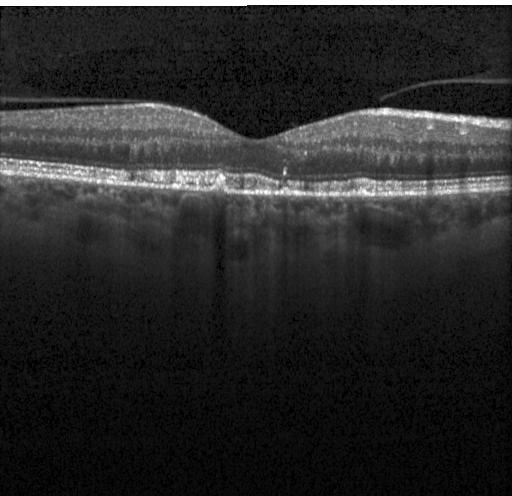
Acquired on a Heidelberg Spectralis · optical coherence tomography B-scan · spectral-domain optical coherence tomography
Finding: multiple drusen.